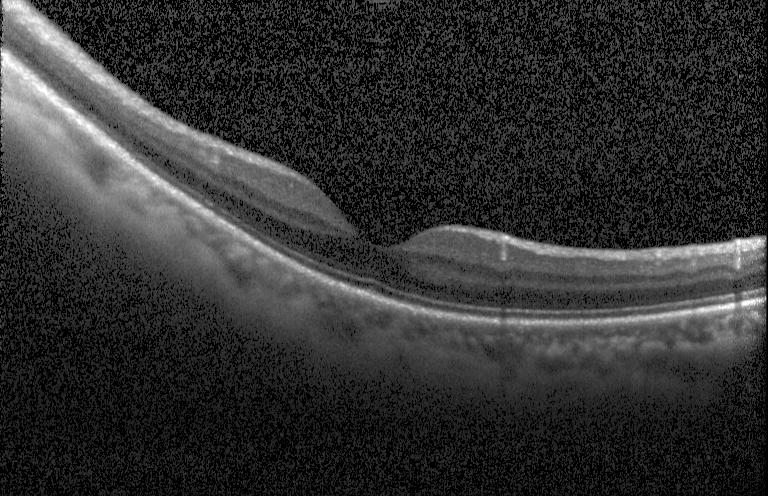 OCT line scan.
No choroidal neovascularization, no diabetic macular edema, and no drusen.